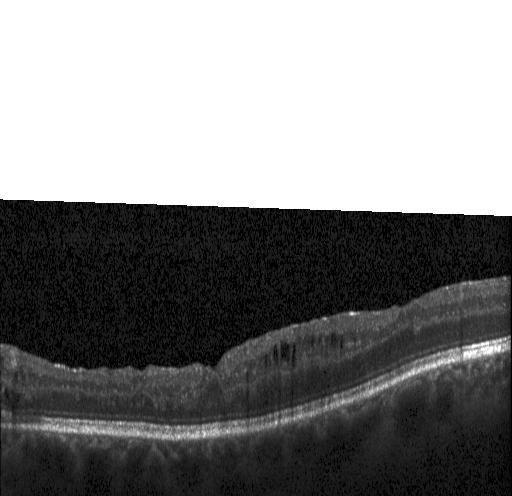 Retinal OCT cross-section; horizontal scan through the fovea.
Finding: diabetic macular edema (DME).